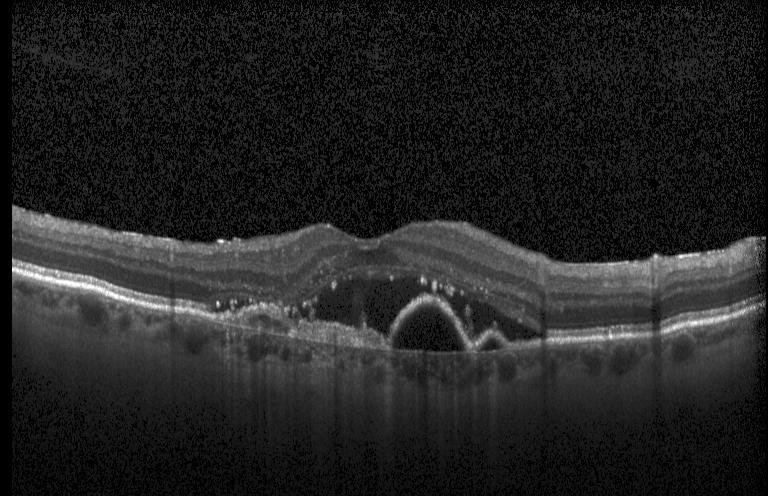
OCT finding: CNV.